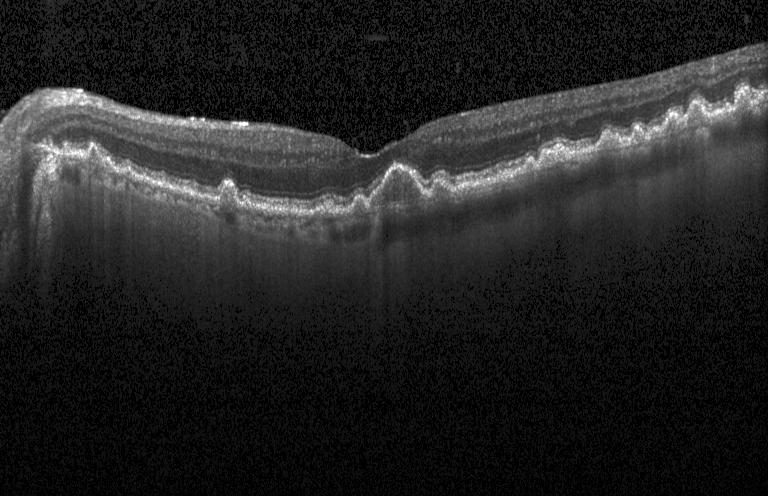
Dx: sub-RPE drusenoid deposits.